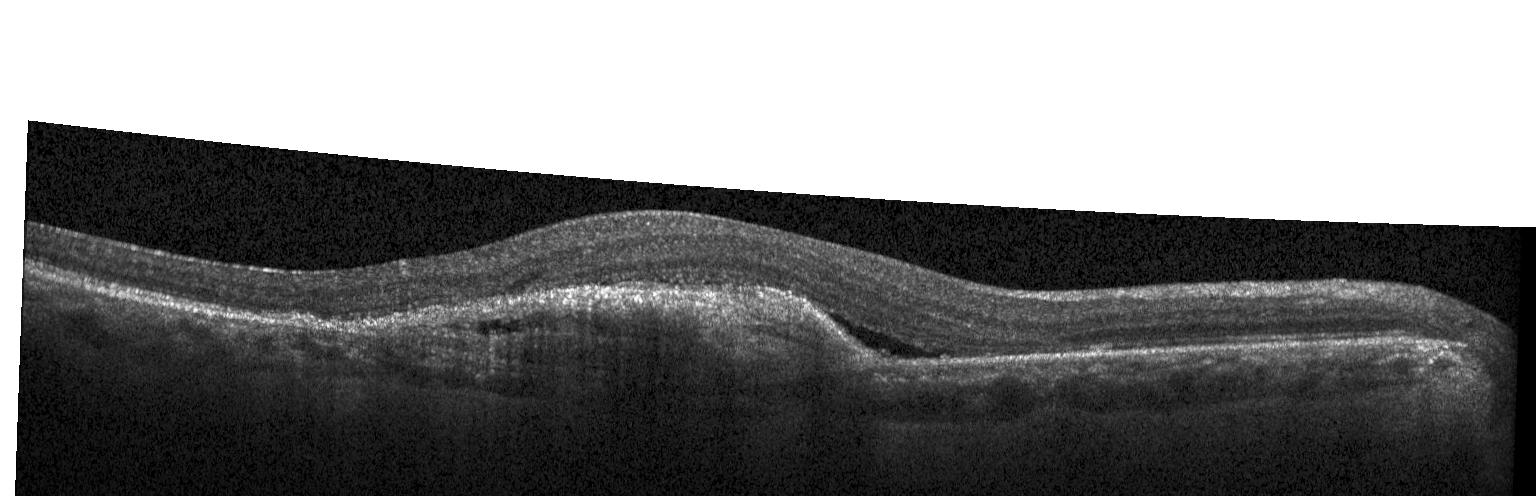 Impression: a choroidal neovascular membrane.